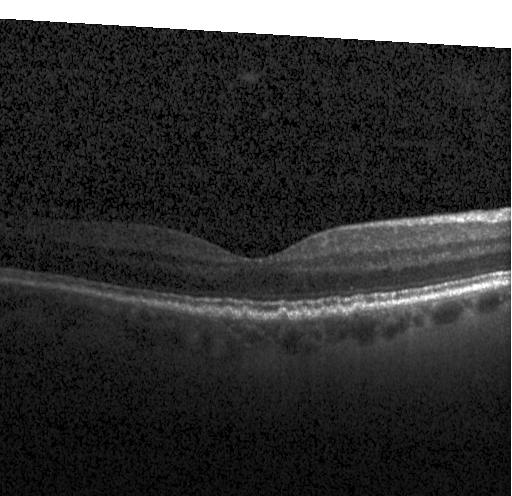
OCT finding: drusen.